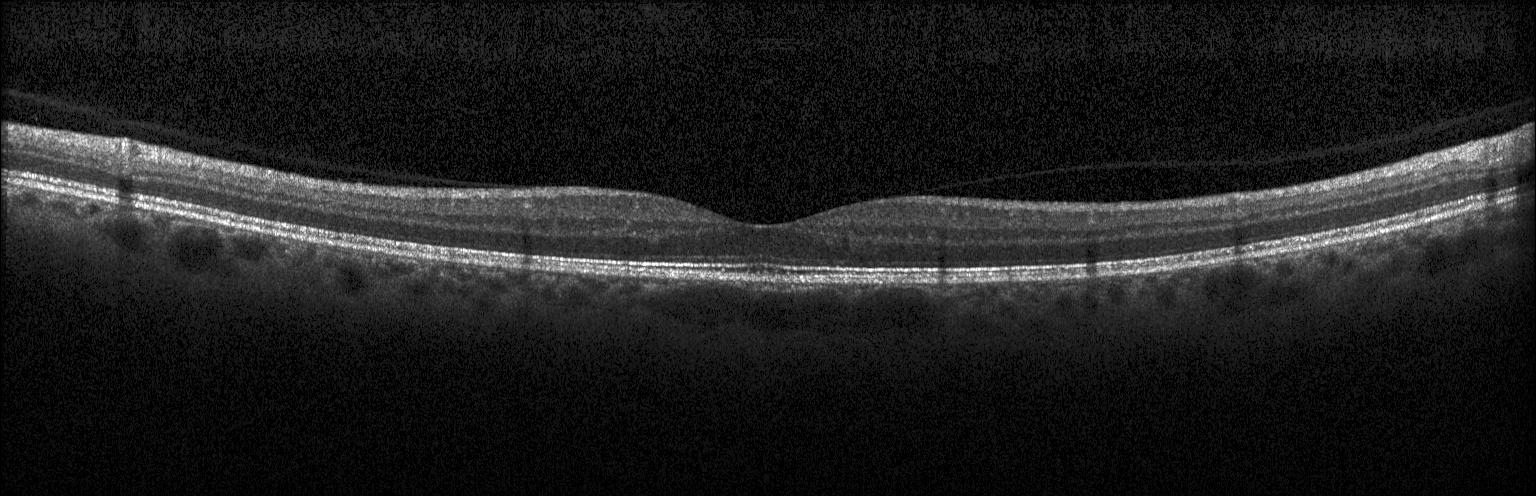

Acquired on a Heidelberg Spectralis, retinal OCT B-scan, spectral-domain optical coherence tomography — Dx: no CNV, no DME, and no drusen.